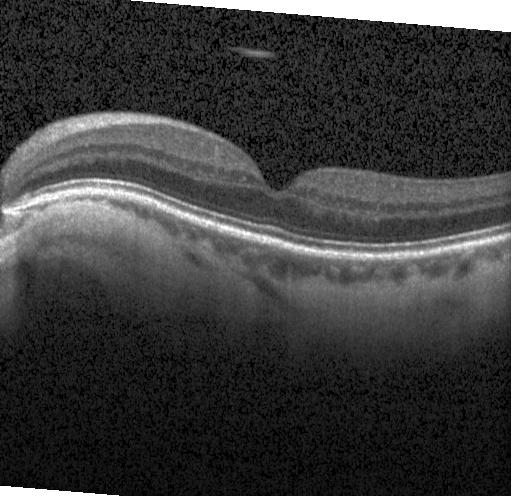

OCT line scan · Heidelberg Spectralis · through the macula.
Diagnosis: neither CNV, DME, nor drusen.